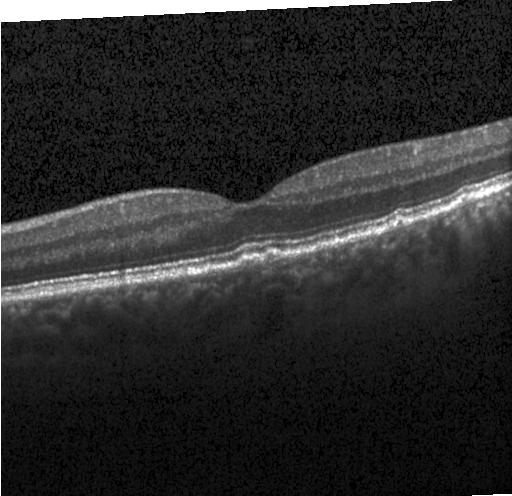 Optical coherence tomography B-scan — Finding: drusen.